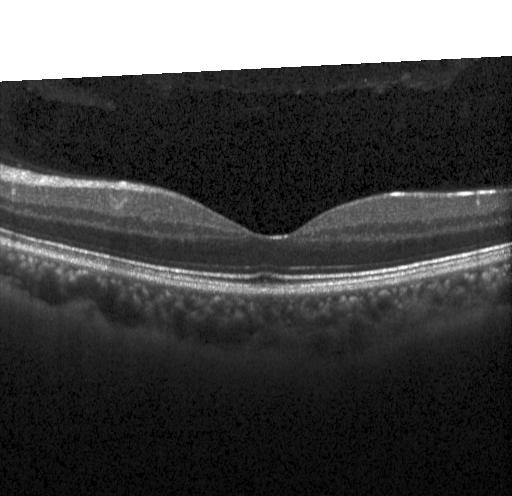
Diagnosis: no choroidal neovascularization, no diabetic macular edema, and no drusen.